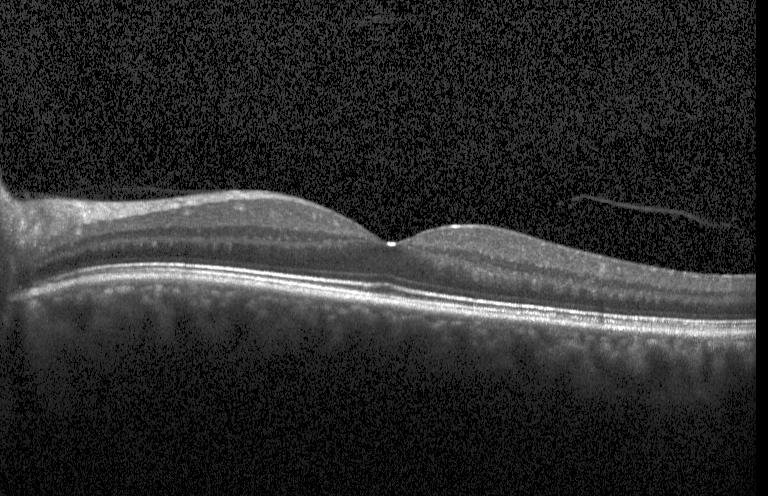 Through the macula, acquired on a Heidelberg Spectralis, spectral-domain OCT, optical coherence tomography B-scan
No choroidal neovascularization, no diabetic macular edema, and no drusen.